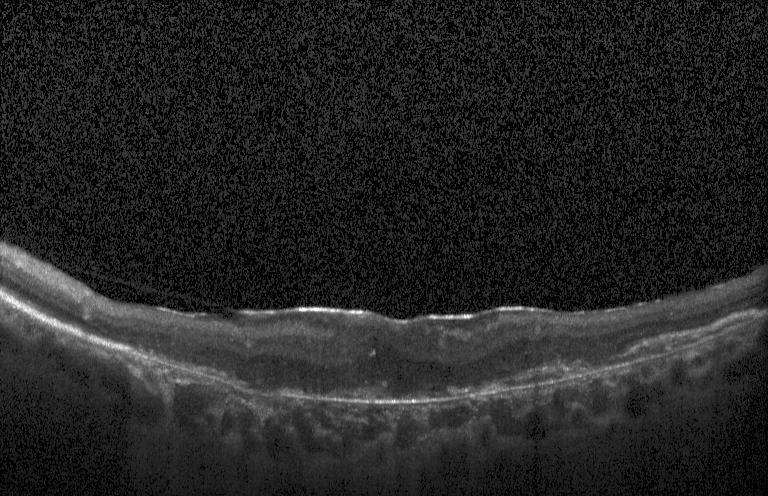 Diagnosis: choroidal neovascularization (CNV).